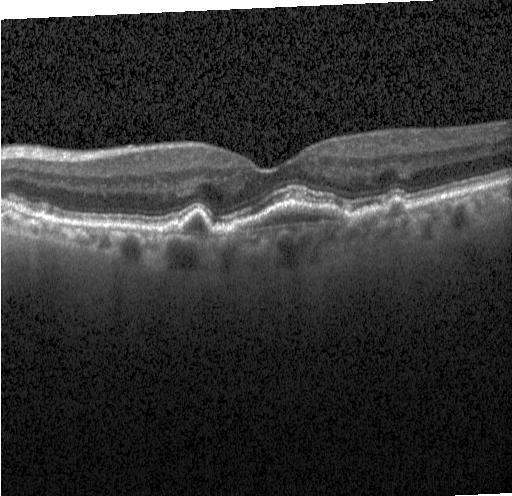

Retinal OCT B-scan · Heidelberg Spectralis OCT system. Impression: a choroidal neovascular membrane.